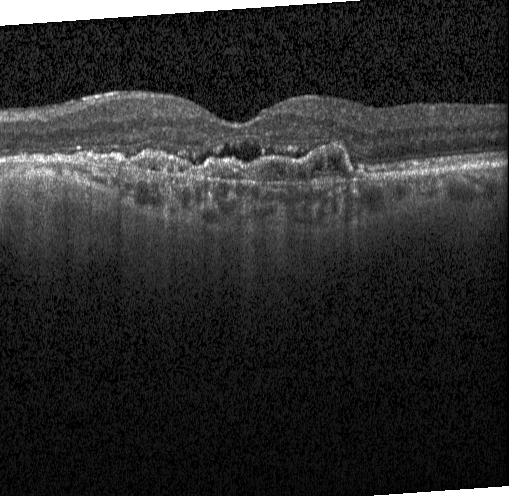
Heidelberg Spectralis. Retinal OCT cross-section. Dx: choroidal neovascularization (CNV).